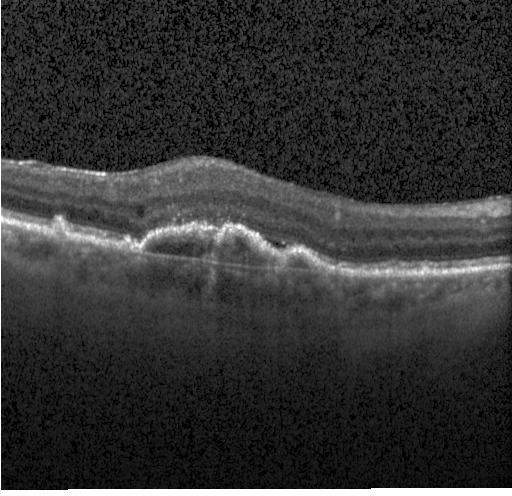
Spectral-domain optical coherence tomography; optical coherence tomography B-scan.
Dx: a choroidal neovascular membrane.